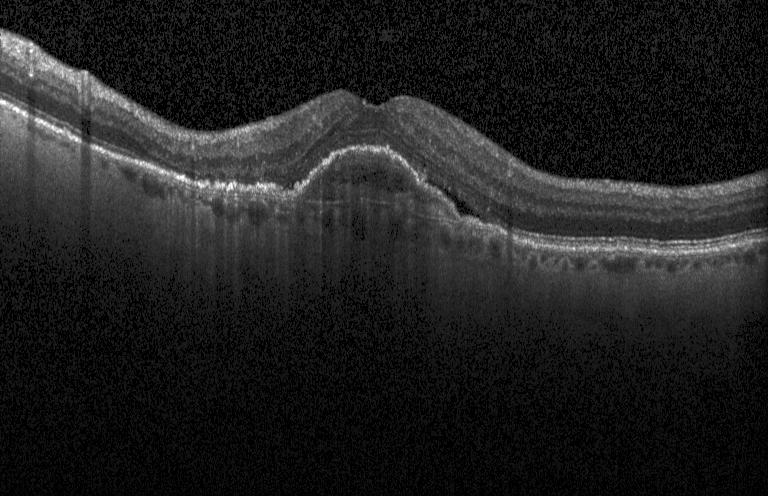

Retinal OCT B-scan — Dx: a choroidal neovascular membrane.